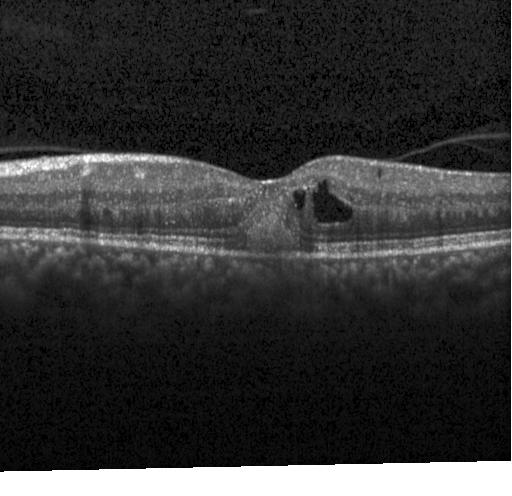

Horizontal scan through the fovea; retinal OCT B-scan; SD-OCT; Heidelberg Spectralis
Impression: a choroidal neovascular membrane.